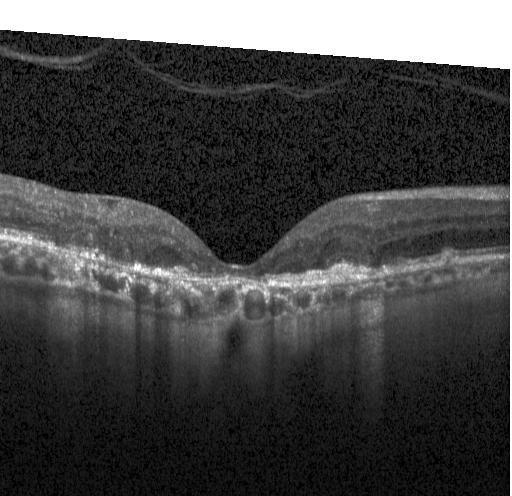
Retinal OCT cross-section. Acquired on a Heidelberg Spectralis.
Impression: a choroidal neovascular membrane.